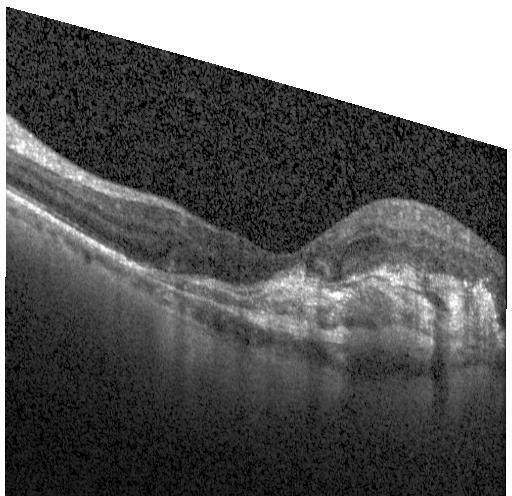
Heidelberg Spectralis · OCT B-scan. Diagnosis: a choroidal neovascular membrane.